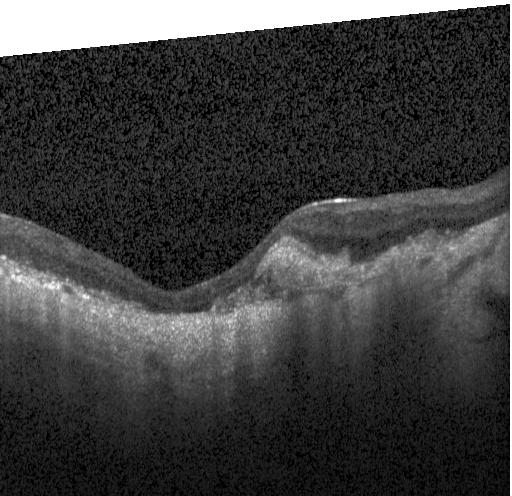

Spectral-domain optical coherence tomography; retinal OCT B-scan; Heidelberg Spectralis OCT system; horizontal scan through the fovea — The scan shows a choroidal neovascular membrane.